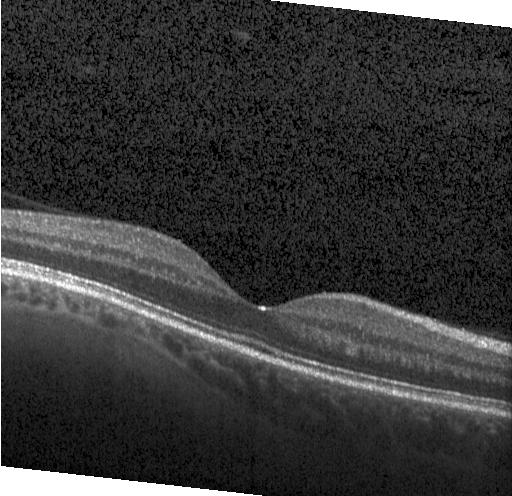
Impression: no evidence of CNV, DME, or drusen.